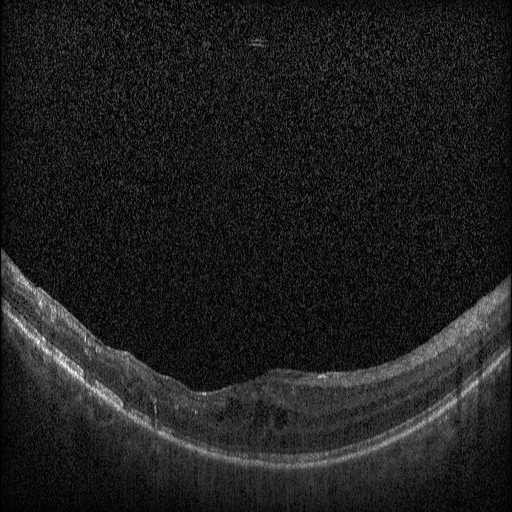
Optical coherence tomography scan · spectral-domain OCT · Heidelberg Spectralis. Finding: diabetic macular edema (DME).